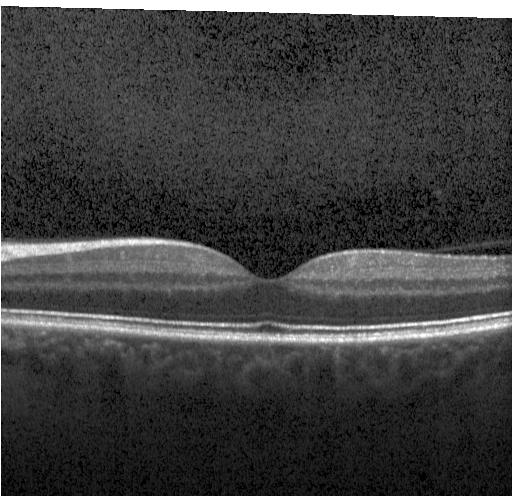

Assessment: no choroidal neovascularization, no diabetic macular edema, and no drusen.